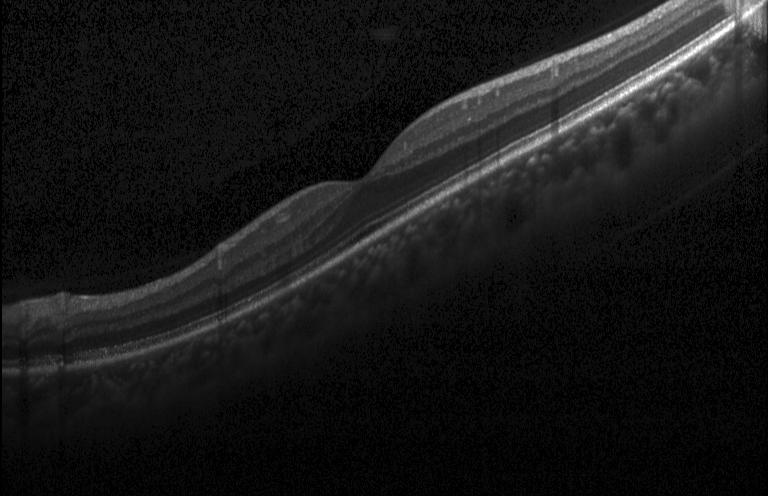 Optical coherence tomography B-scan. Spectral-domain OCT. Macular scan. Heidelberg Spectralis OCT system.
Dx: no evidence of CNV, DME, or drusen.